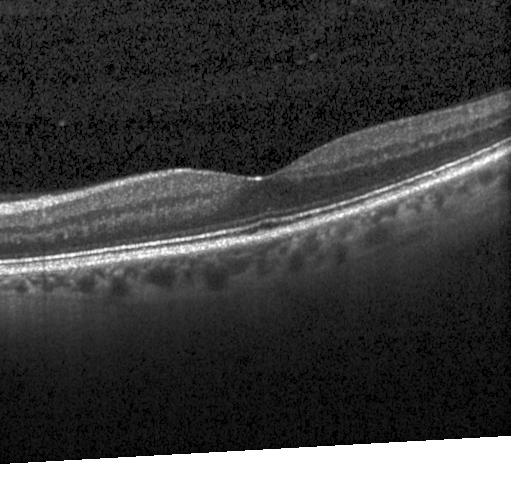
Retinal OCT cross-section. Through the macula. Instrument: Heidelberg Spectralis. Spectral-domain OCT. This B-scan demonstrates no CNV, no DME, and no drusen.